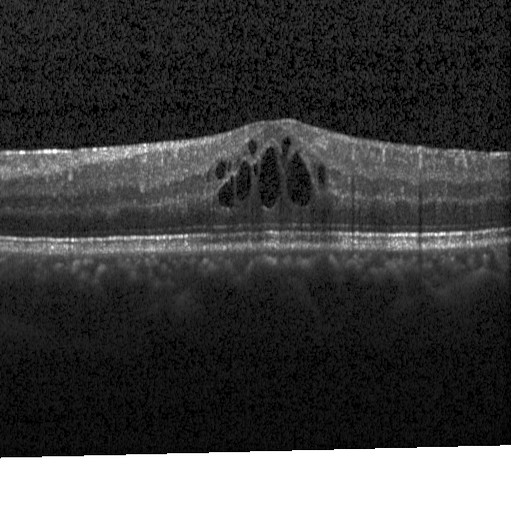

Optical coherence tomography scan — Impression: DME.